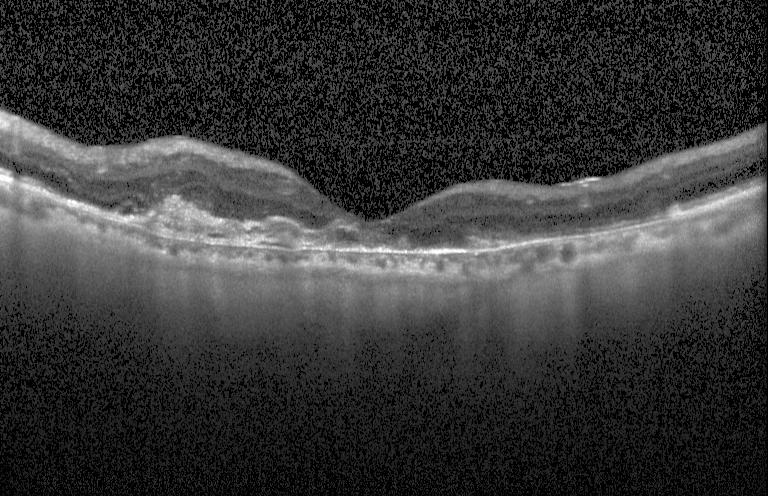 OCT B-scan. Centered on the fovea. Instrument: Heidelberg Spectralis. SD-OCT. Finding: a choroidal neovascular membrane.